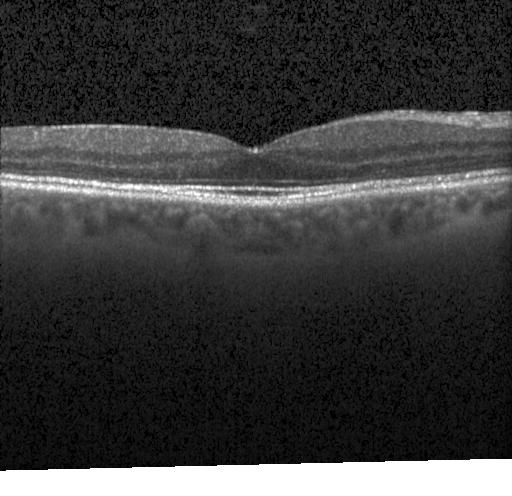
Through the macula, spectral-domain optical coherence tomography, optical coherence tomography scan. Diagnosis: no choroidal neovascularization, diabetic macular edema, or drusen.